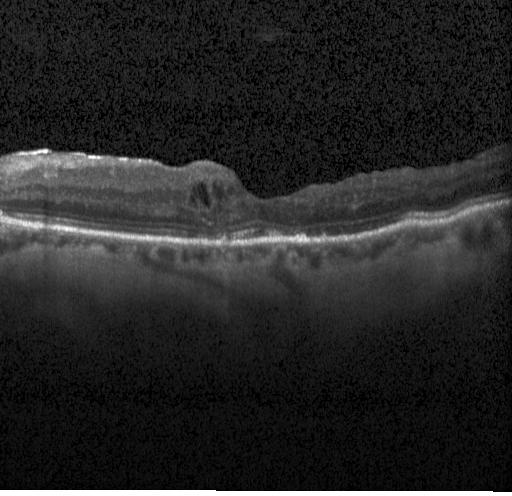

Macular OCT: diabetic macular edema.